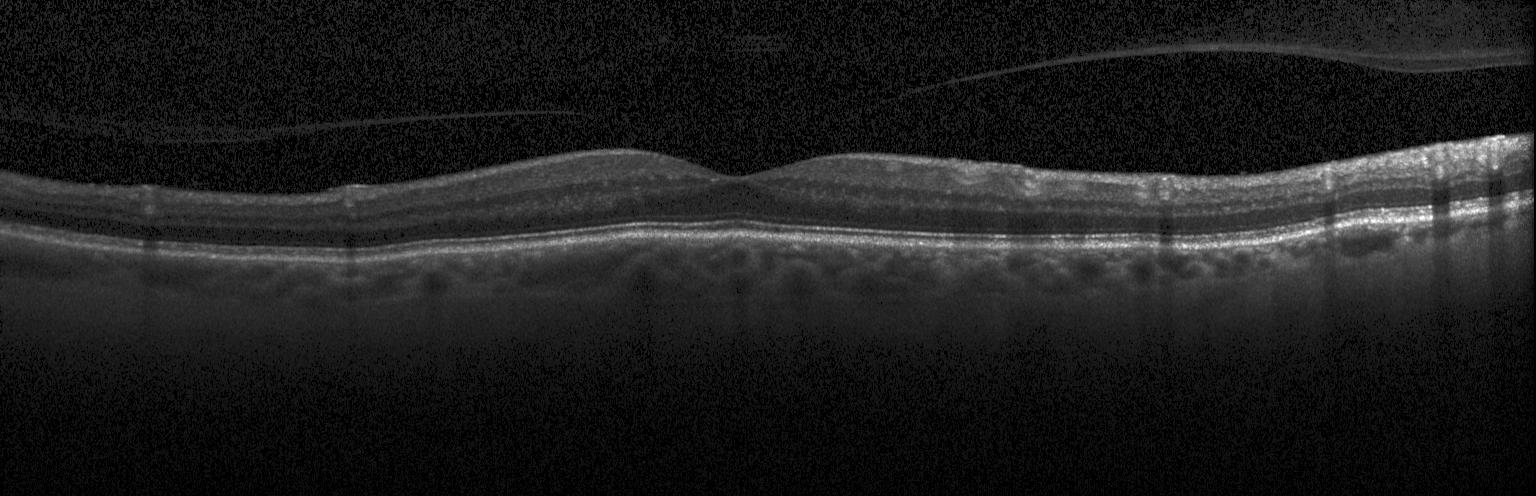

Diagnosis: no evidence of choroidal neovascularization, diabetic macular edema, or drusen.